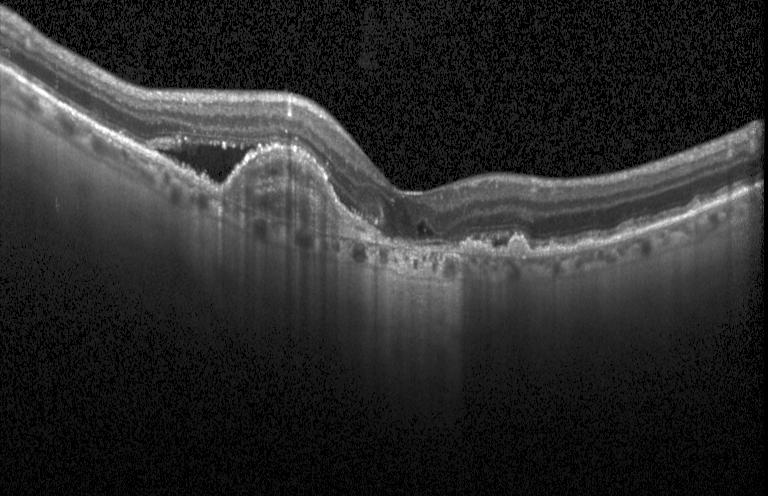
Optical coherence tomography scan — Diagnosis: a choroidal neovascular membrane.